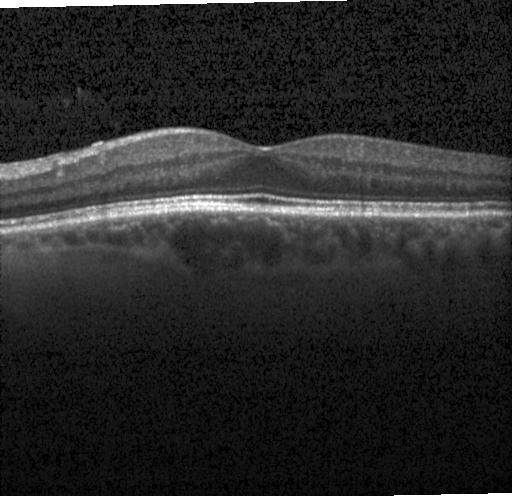
Diagnosis: no choroidal neovascularization, no diabetic macular edema, and no drusen.